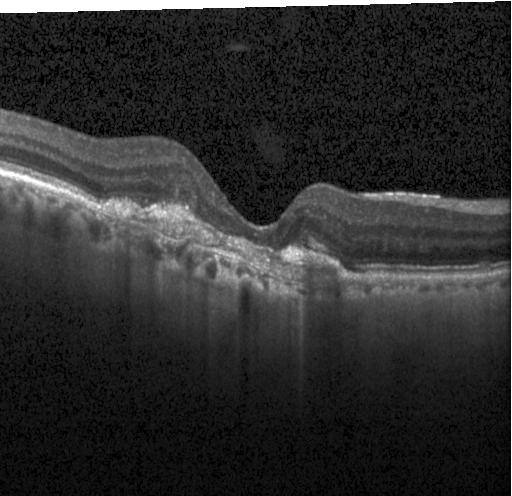
Through the macula. Optical coherence tomography scan. Spectral-domain OCT — Macular OCT: CNV.